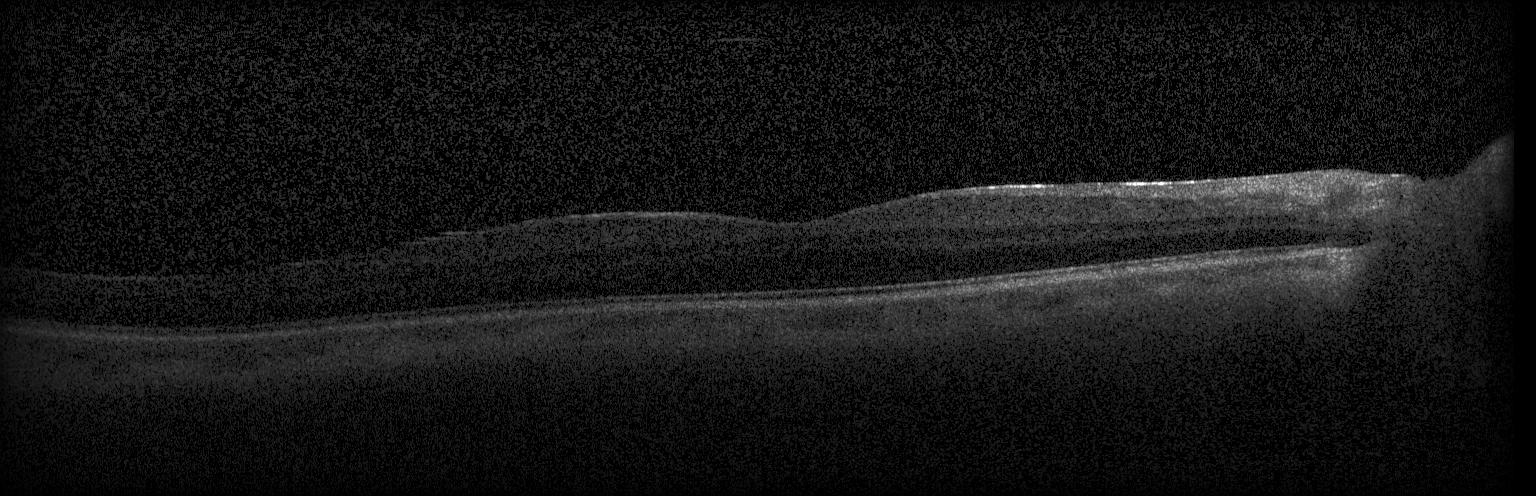 OCT line scan
Impression: no evidence of choroidal neovascularization, diabetic macular edema, or drusen.